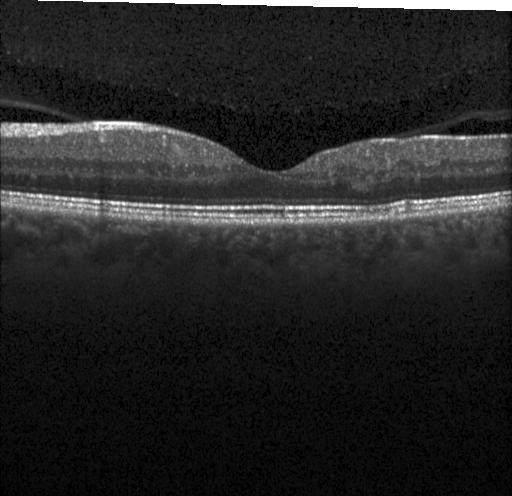 Retinal OCT cross-section, Heidelberg Spectralis OCT system. Assessment: neither CNV, DME, nor drusen.